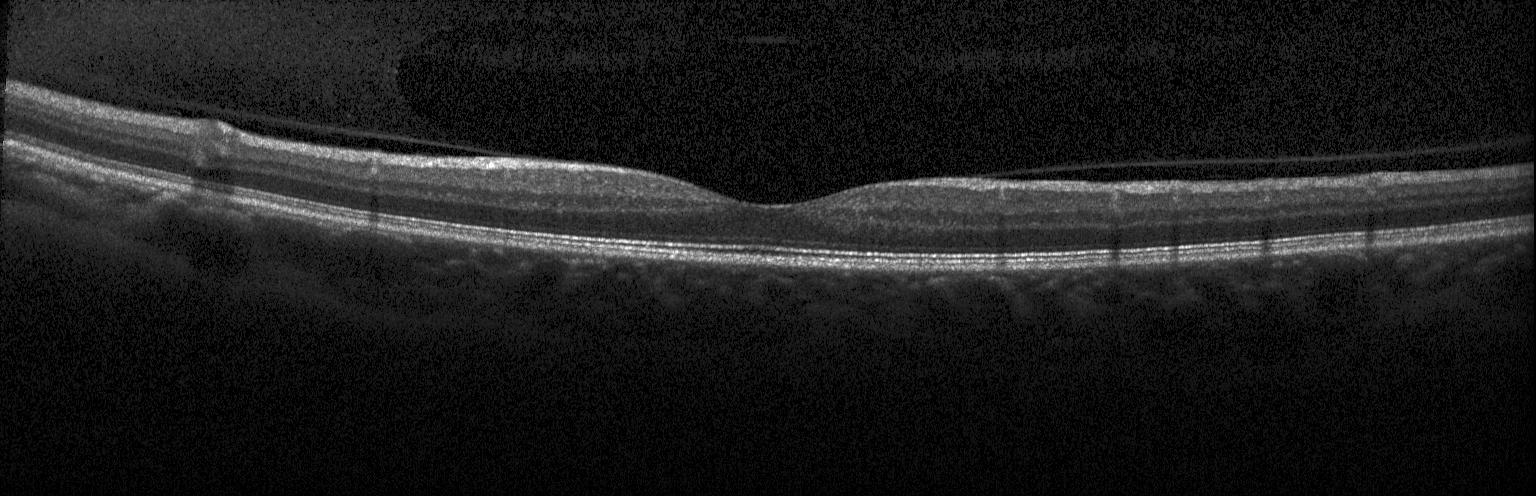 OCT B-scan.
Finding: no choroidal neovascularization, no diabetic macular edema, and no drusen.